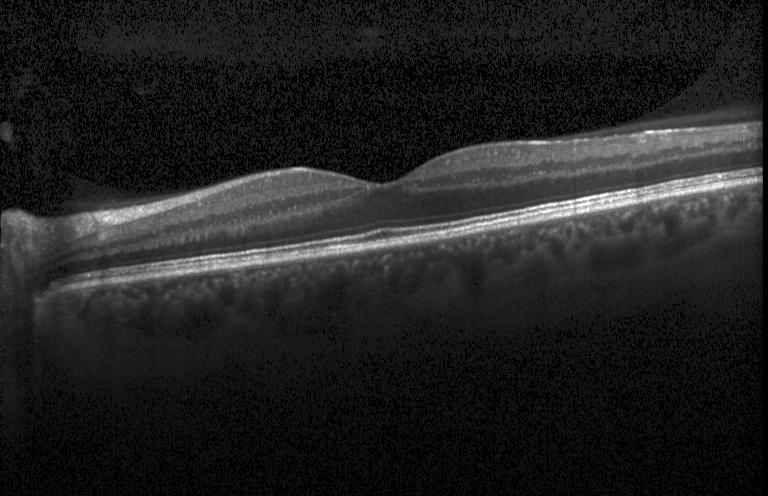 Fovea-centered · OCT B-scan · acquired on a Heidelberg Spectralis · SD-OCT — Dx: no choroidal neovascularization, no diabetic macular edema, and no drusen.